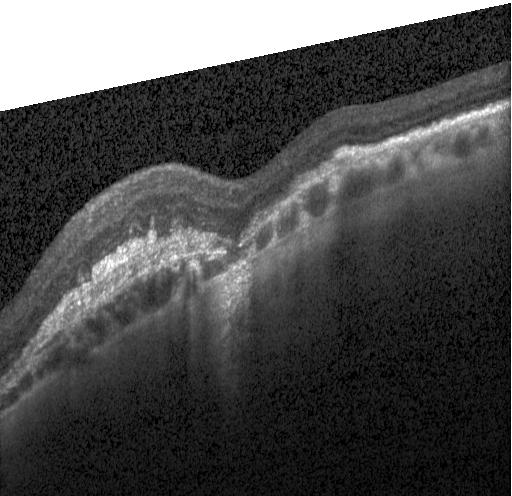 A choroidal neovascular membrane.